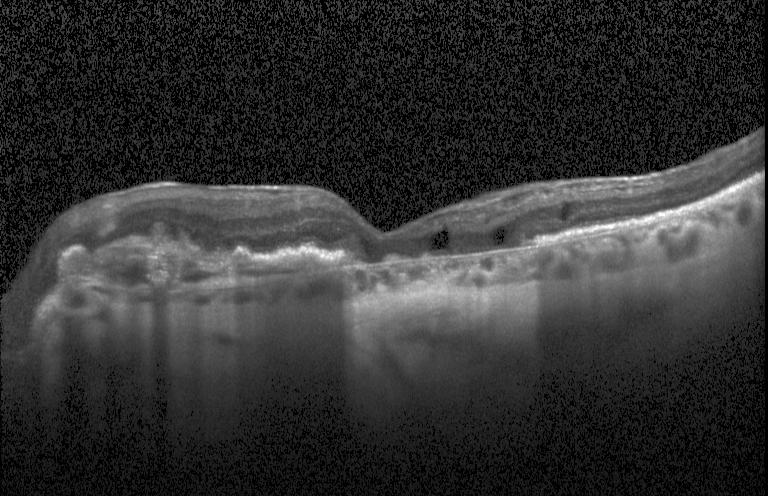

Retinal OCT B-scan, acquired on a Heidelberg Spectralis
Assessment: choroidal neovascularization (CNV).